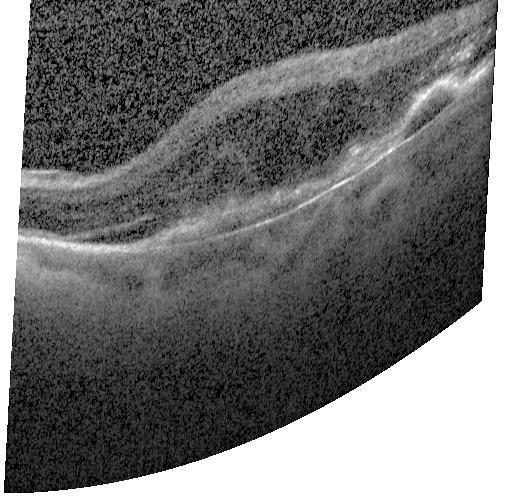

Retinal OCT B-scan, SD-OCT. Diagnosis: a choroidal neovascular membrane.